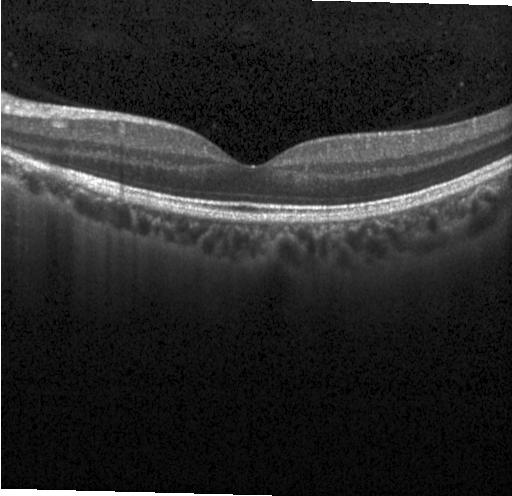

SD-OCT. Heidelberg Spectralis. OCT B-scan. No evidence of choroidal neovascularization, diabetic macular edema, or drusen.